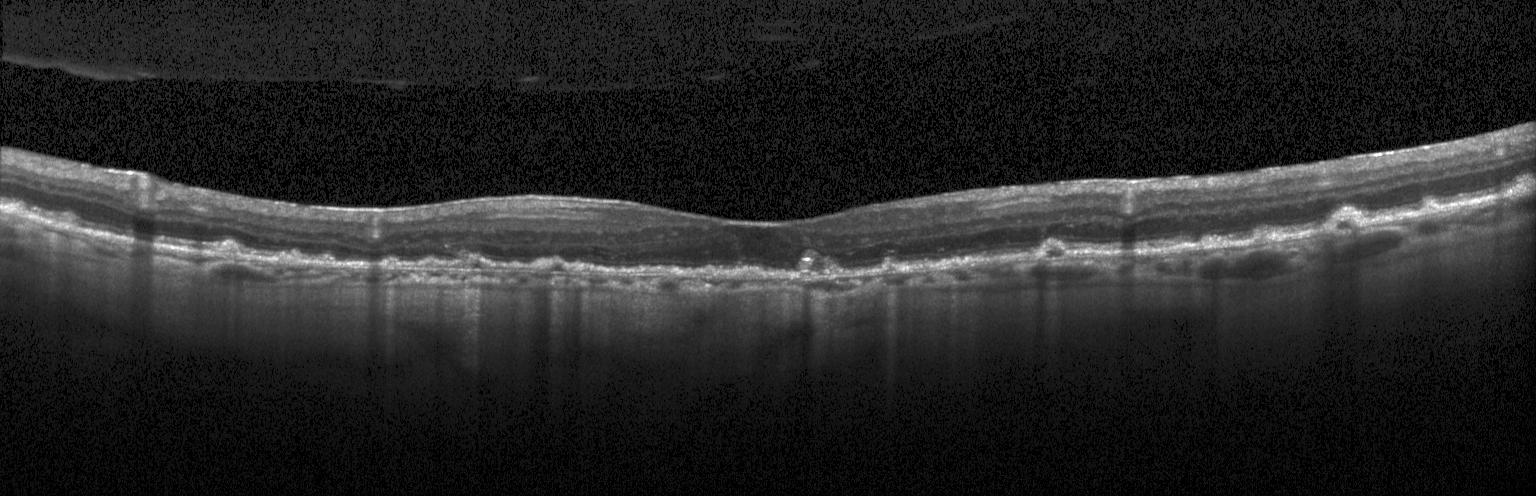

Retinal OCT B-scan.
Choroidal neovascularization (CNV).